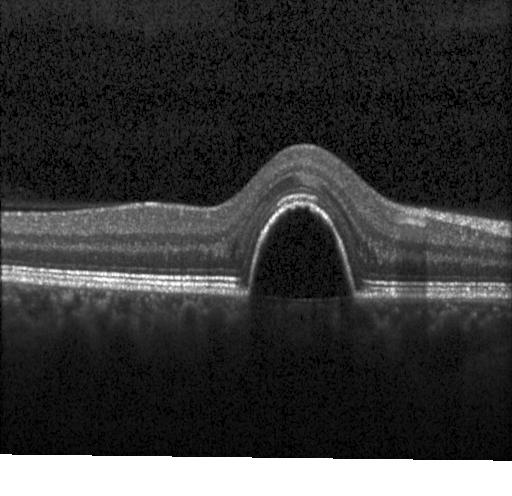 Diagnosis: choroidal neovascularization.